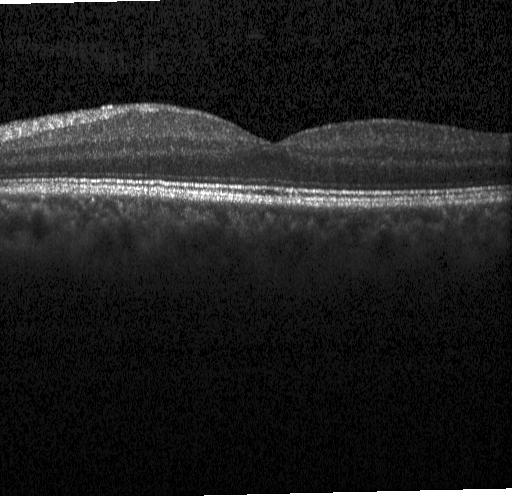 Optical coherence tomography B-scan · macular scan · spectral-domain optical coherence tomography.
Dx: no choroidal neovascularization, no diabetic macular edema, and no drusen.